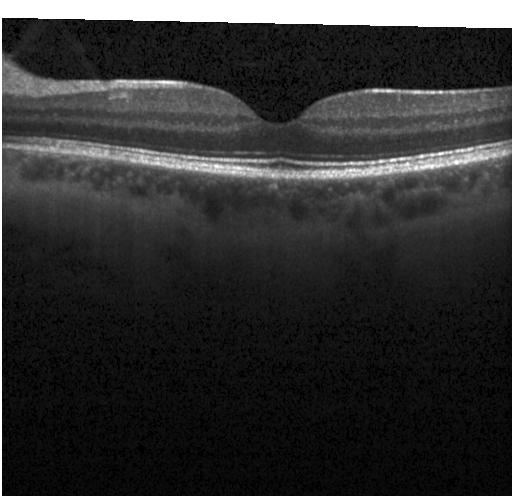

Retinal OCT B-scan · Heidelberg Spectralis
Impression: no choroidal neovascularization, no diabetic macular edema, and no drusen.